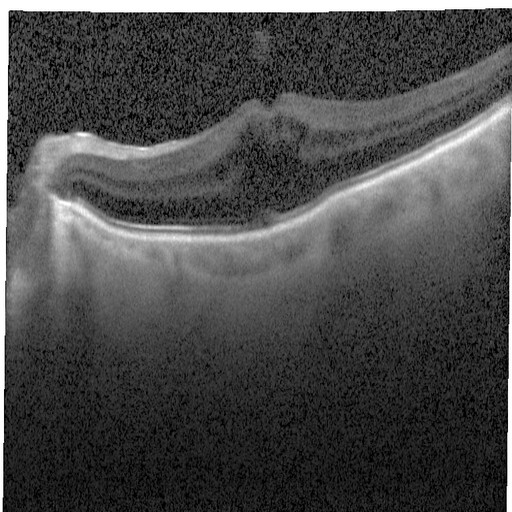
Optical coherence tomography B-scan; acquired on a Heidelberg Spectralis; macular scan; SD-OCT
Dx: diabetic macular edema (DME).